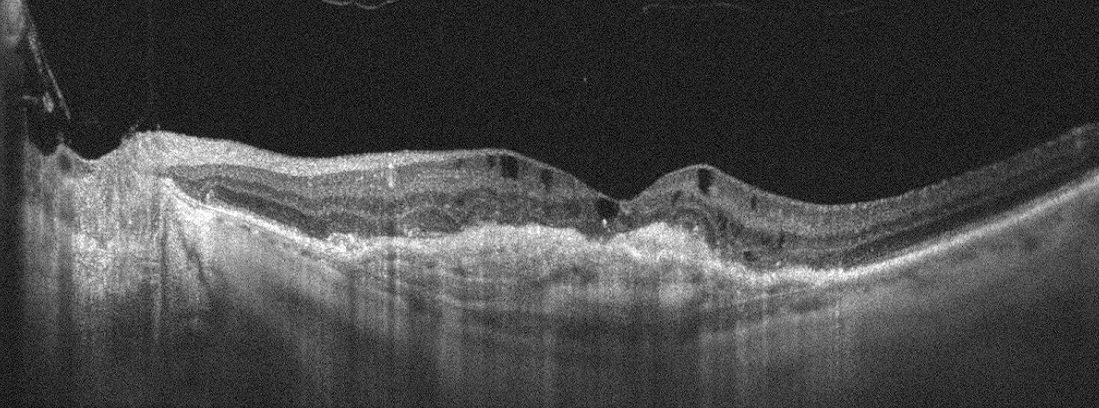 Finding: age-related macular degeneration.